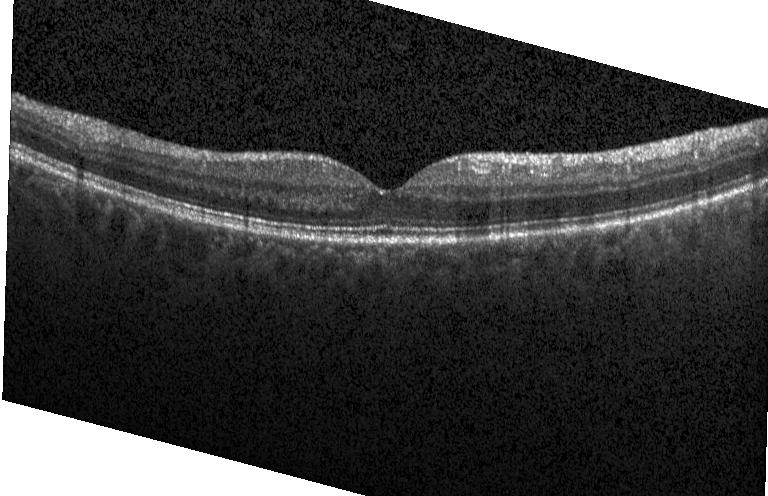

Impression: neither choroidal neovascularization, diabetic macular edema, nor drusen.